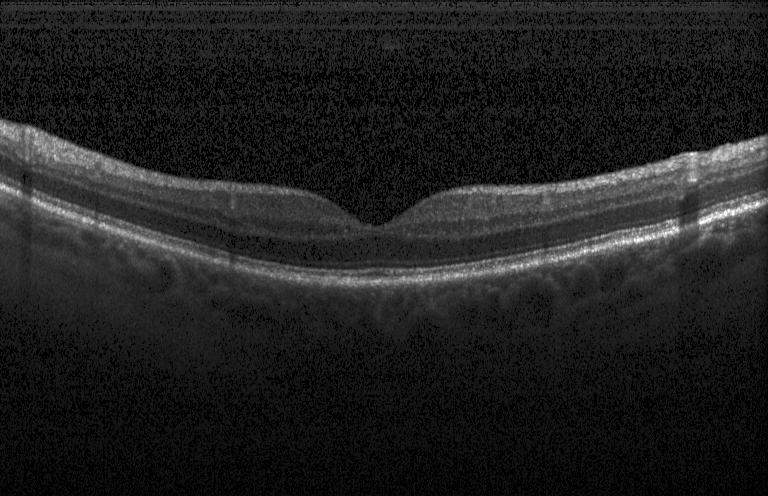
Macular OCT: no choroidal neovascularization, diabetic macular edema, or drusen.